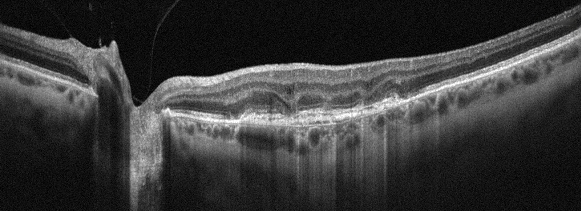

Left eye, OCT line scan, fovea-centered.
This B-scan demonstrates AMD.